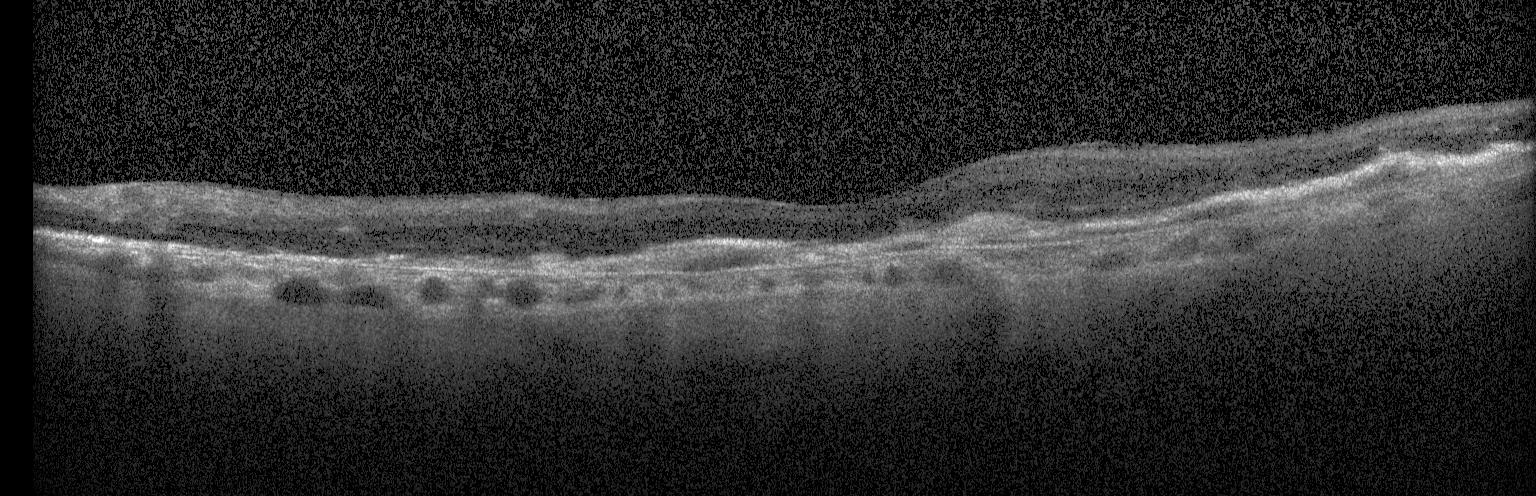
Spectral-domain OCT; optical coherence tomography B-scan; acquired on a Heidelberg Spectralis
This B-scan demonstrates a choroidal neovascular membrane.